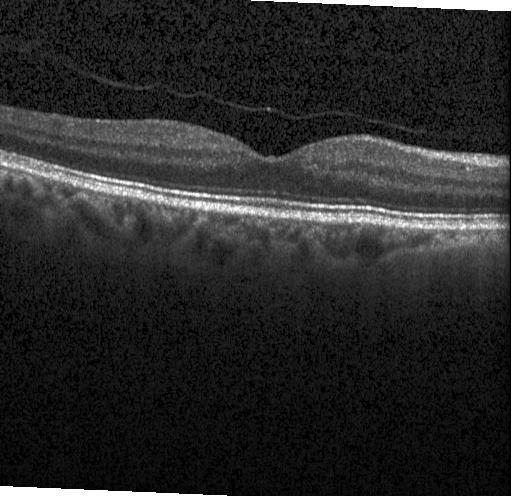

Impression: neither choroidal neovascularization, diabetic macular edema, nor drusen.